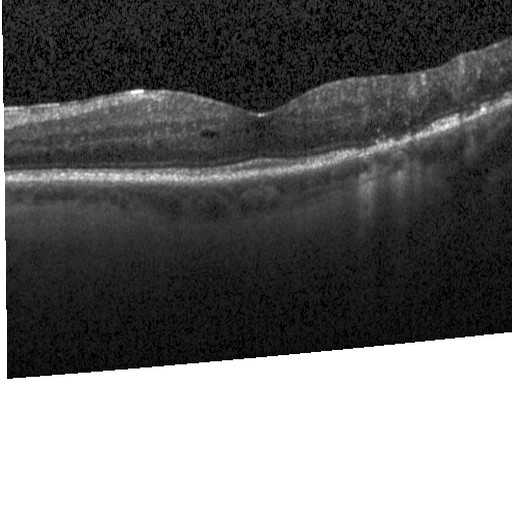

Optical coherence tomography B-scan
The scan shows DME.